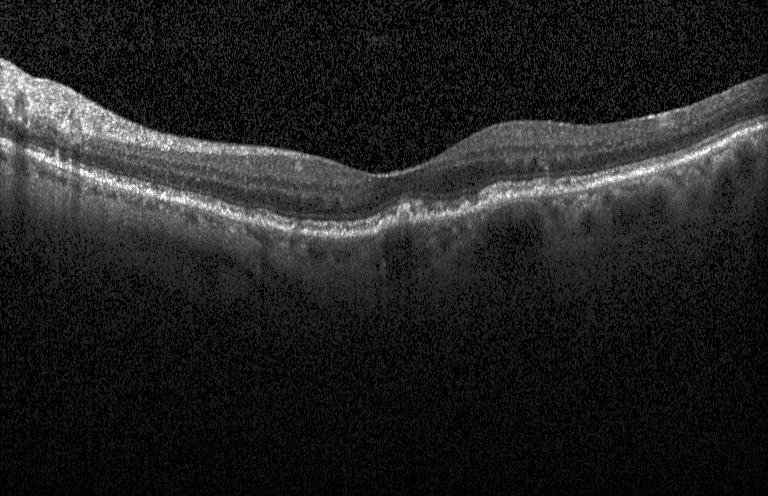

SD-OCT. Heidelberg Spectralis. Optical coherence tomography B-scan.
Multiple drusen.